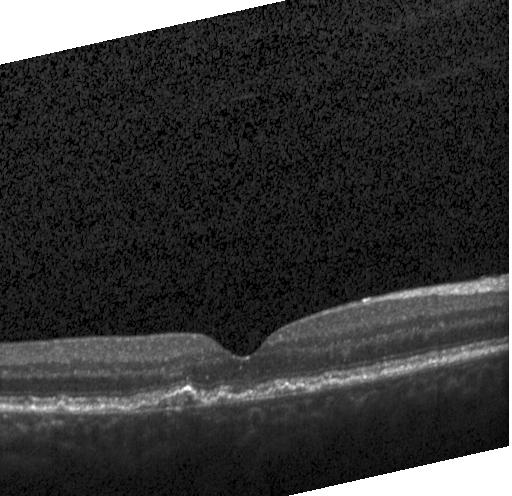 OCT scan showing CNV.